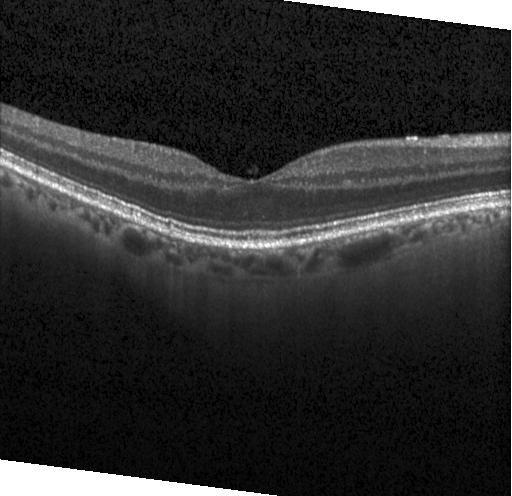 Dx: neither CNV, DME, nor drusen.